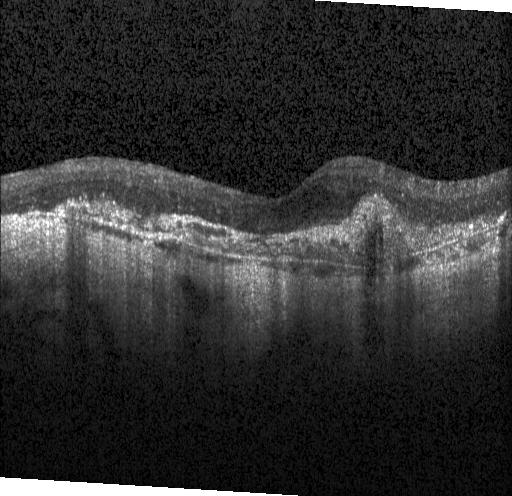

Macular OCT: CNV.